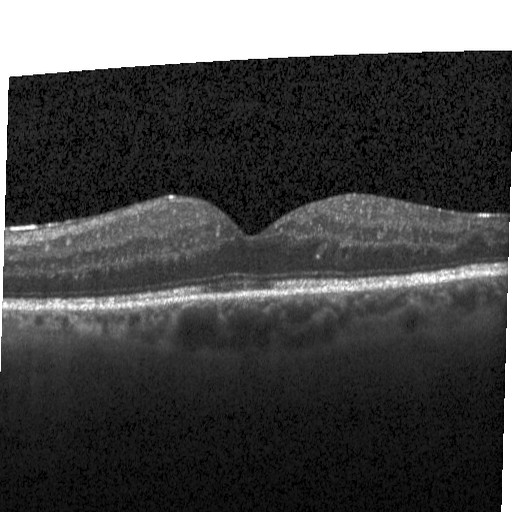
Retinal OCT B-scan.
Finding: diabetic macular edema (DME).